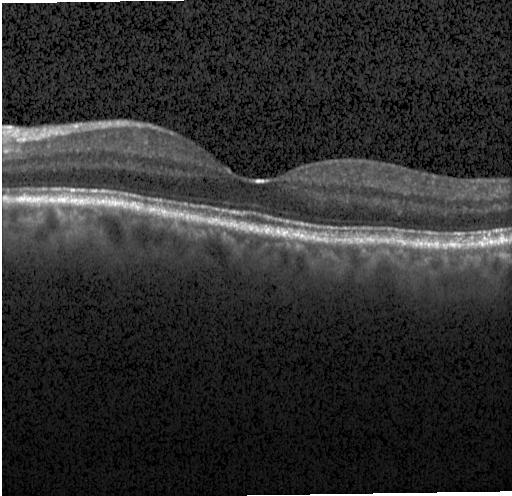

Macular scan; instrument: Heidelberg Spectralis; retinal OCT cross-section; SD-OCT. No choroidal neovascularization, no diabetic macular edema, and no drusen.